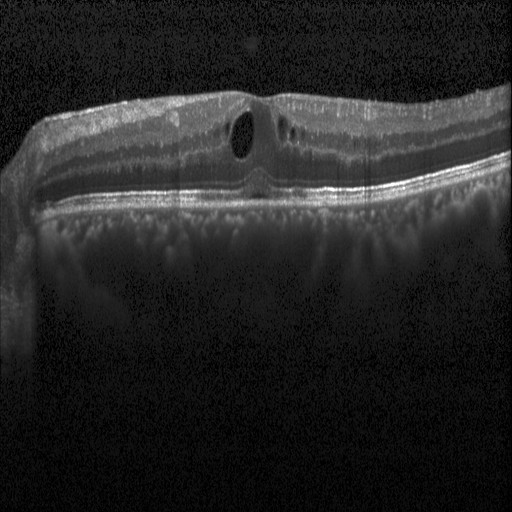

Macular scan · retinal OCT B-scan · spectral-domain optical coherence tomography. Dx: diabetic macular edema (DME).